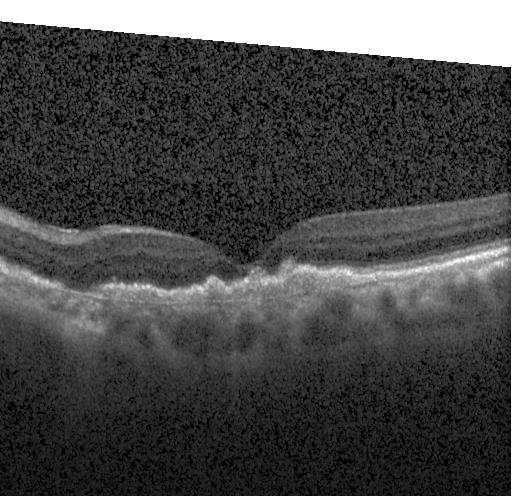

OCT B-scan · centered on the fovea.
The scan shows choroidal neovascularization (CNV).